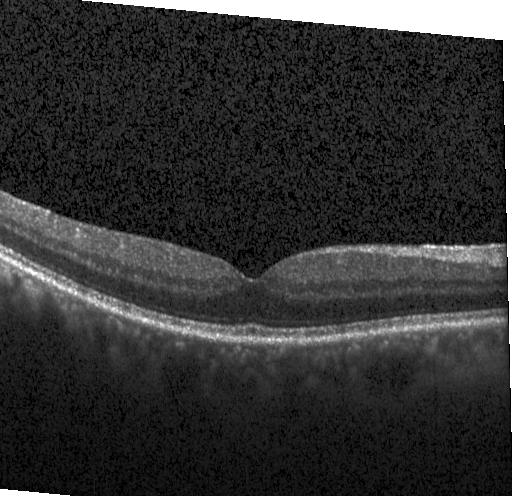

Spectral-domain OCT · horizontal scan through the fovea · optical coherence tomography scan. OCT finding: neither CNV, DME, nor drusen.